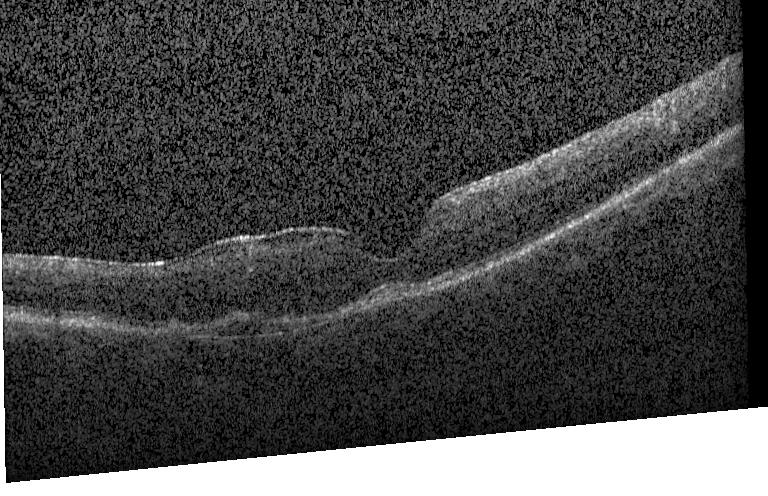

Choroidal neovascularization.